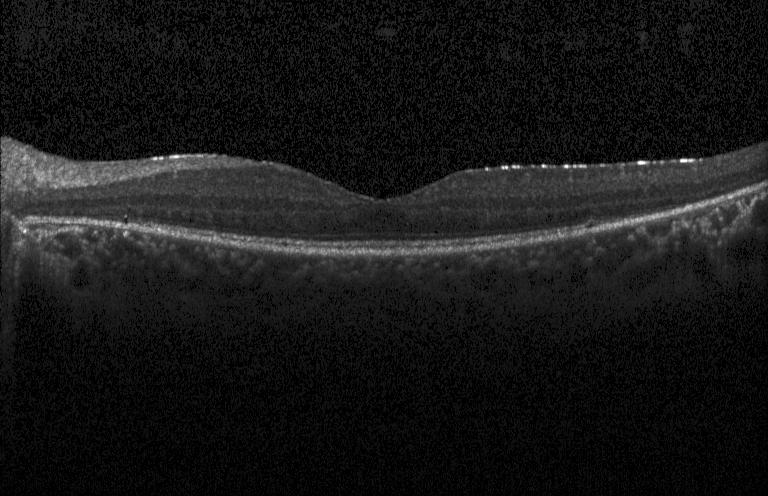 Optical coherence tomography scan. Centered on the fovea. Spectral-domain optical coherence tomography. Finding: no CNV, DME, or drusen.